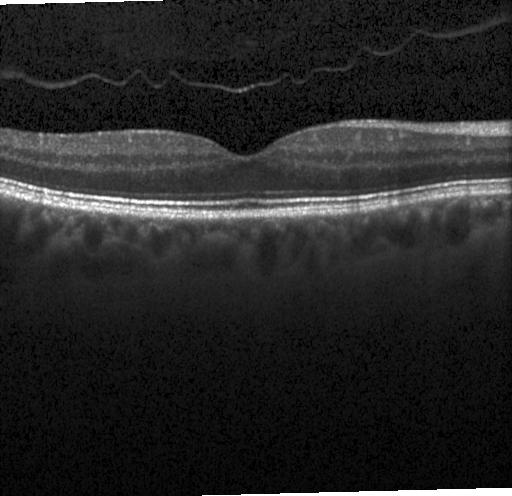

Optical coherence tomography B-scan · fovea-centered · spectral-domain optical coherence tomography · Heidelberg Spectralis OCT system. Diagnosis: no evidence of CNV, DME, or drusen.